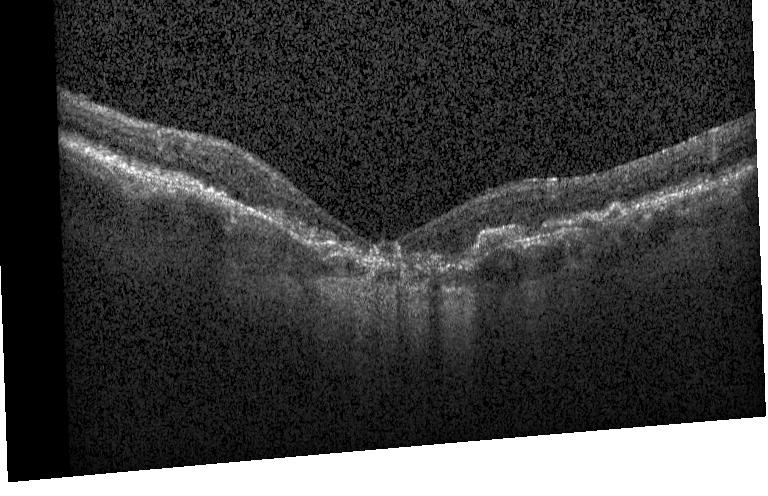 Macular scan · instrument: Heidelberg Spectralis · retinal OCT B-scan · spectral-domain optical coherence tomography.
Diagnosis: choroidal neovascularization.